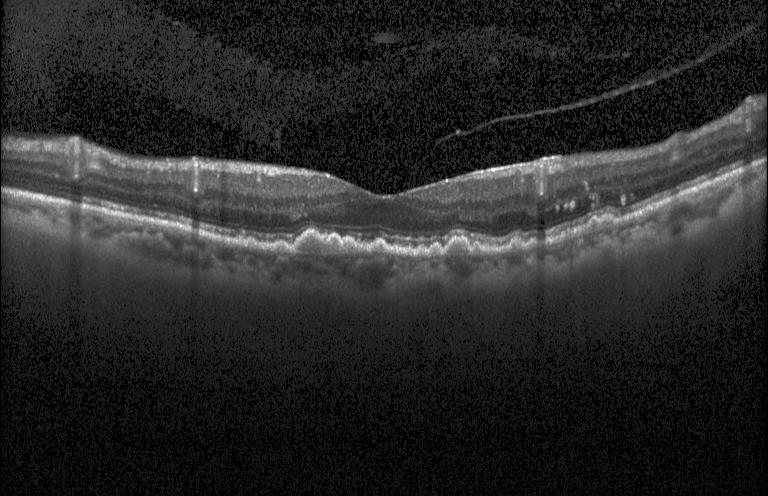

Fovea-centered. Optical coherence tomography B-scan
Finding: choroidal neovascularization.